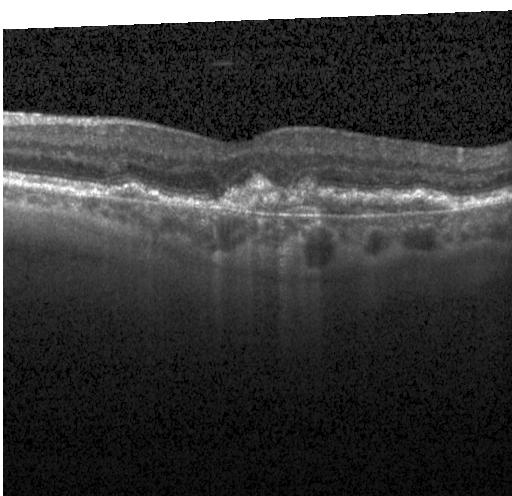
Spectral-domain optical coherence tomography; retinal OCT B-scan; macular scan
Impression: choroidal neovascularization (CNV).